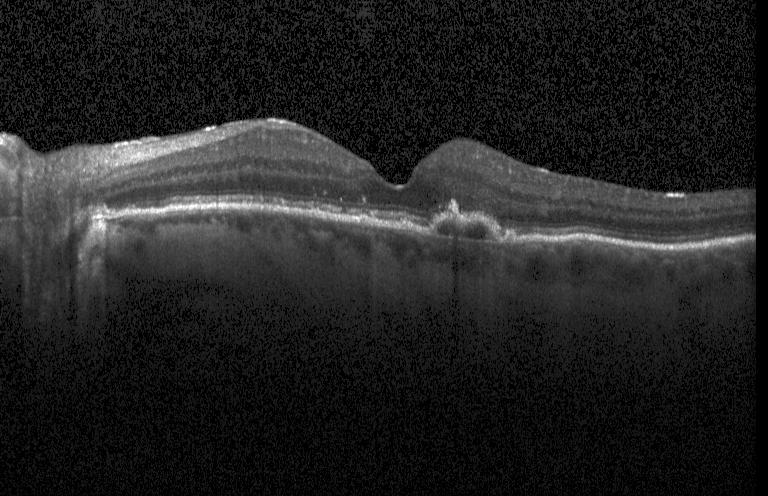

Horizontal scan through the fovea · optical coherence tomography B-scan · spectral-domain optical coherence tomography.
This B-scan demonstrates a choroidal neovascular membrane.